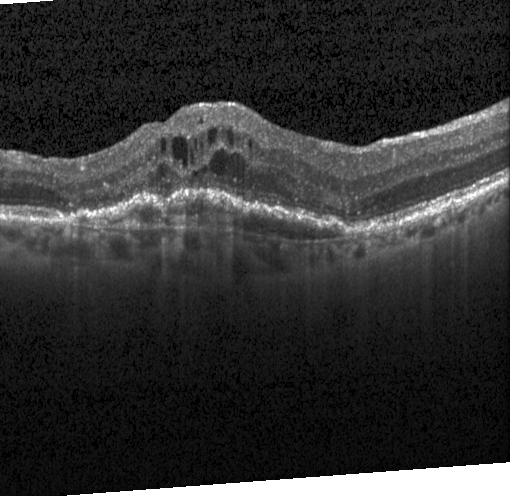 Diagnosis: a choroidal neovascular membrane.